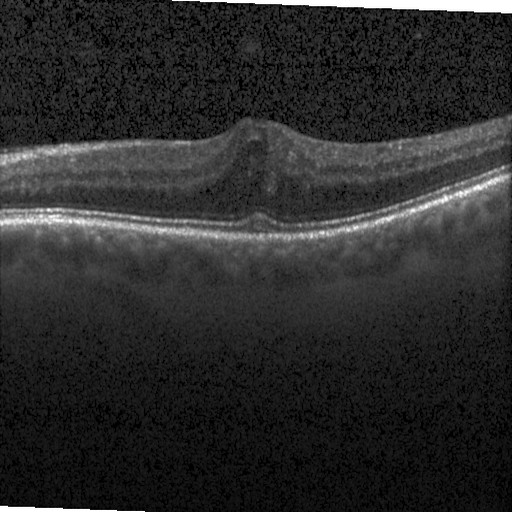
Spectral-domain OCT B-scan: diabetic macular edema (DME).